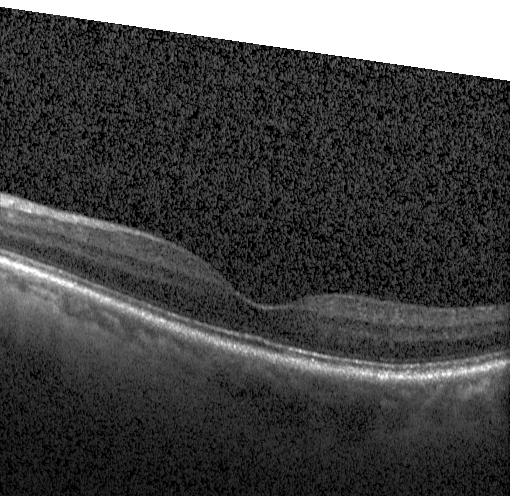 Horizontal scan through the fovea. Spectral-domain OCT. Retinal OCT B-scan.
Impression: neither CNV, DME, nor drusen.